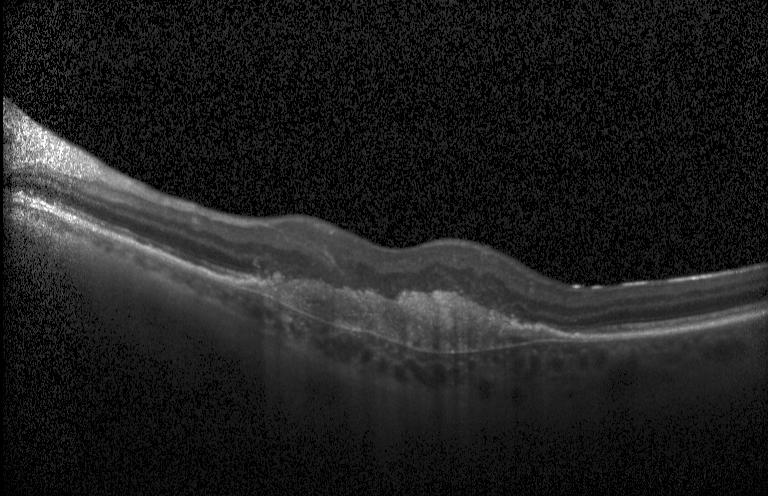

Finding: choroidal neovascularization.